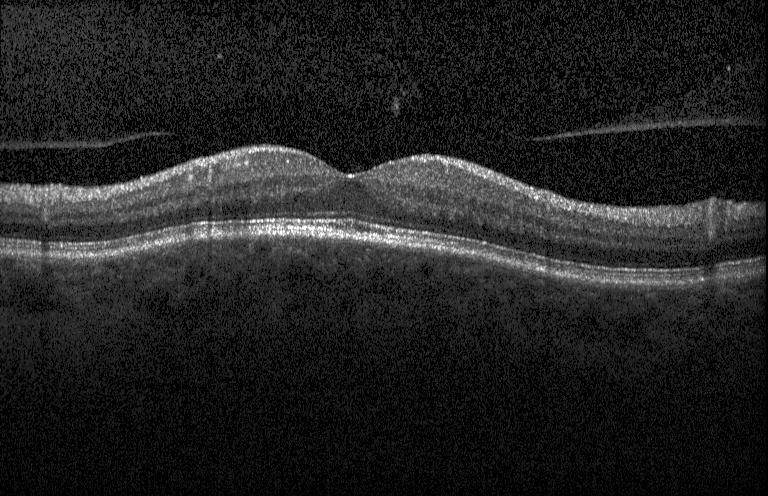 Spectral-domain OCT; optical coherence tomography scan; macular scan
The scan shows neither choroidal neovascularization, diabetic macular edema, nor drusen.